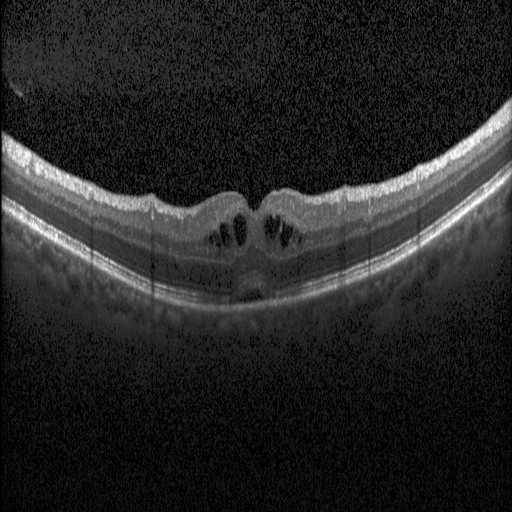 Retinal OCT cross-section · horizontal scan through the fovea · instrument: Heidelberg Spectralis
Finding: diabetic macular edema (DME).